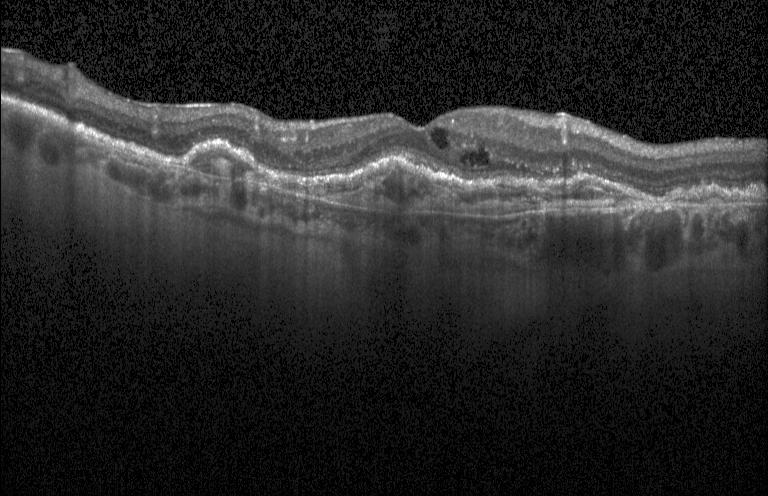 Finding: CNV.